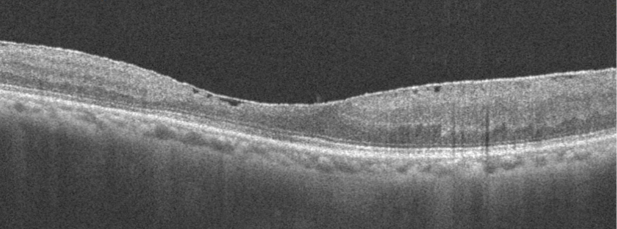

Fovea-centered · optical coherence tomography B-scan
Impression: ERM.